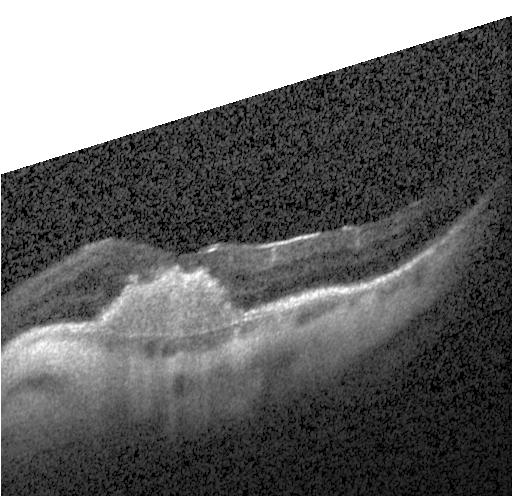 Impression: choroidal neovascularization (CNV).